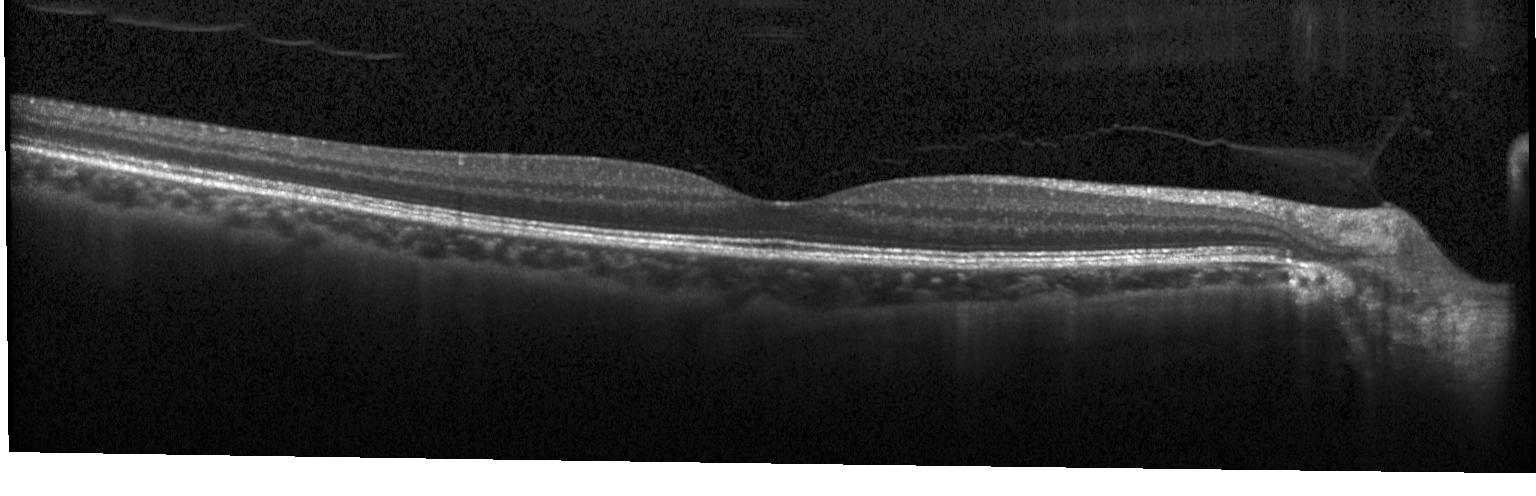 OCT line scan — Assessment: no CNV, no DME, and no drusen.